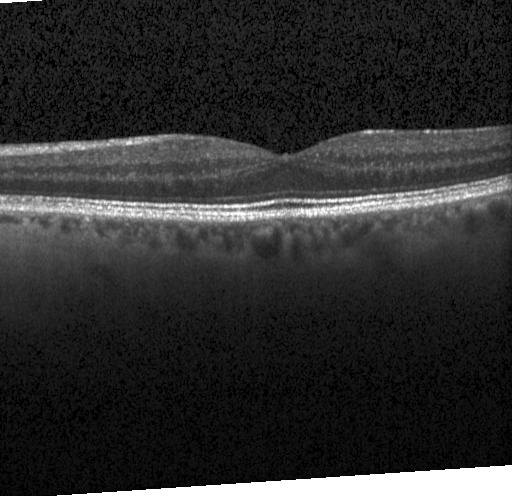
Fovea-centered · OCT B-scan.
Diagnosis: neither CNV, DME, nor drusen.